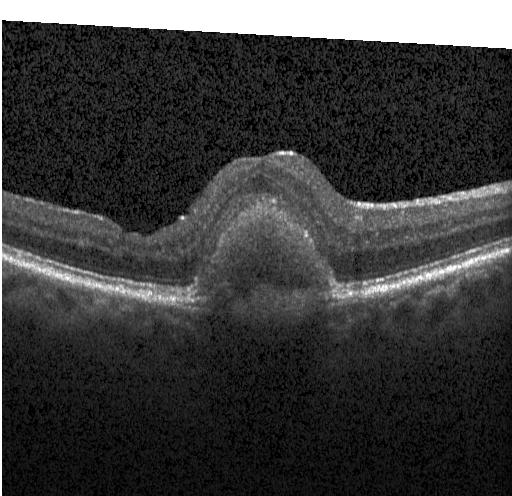 Impression: CNV.